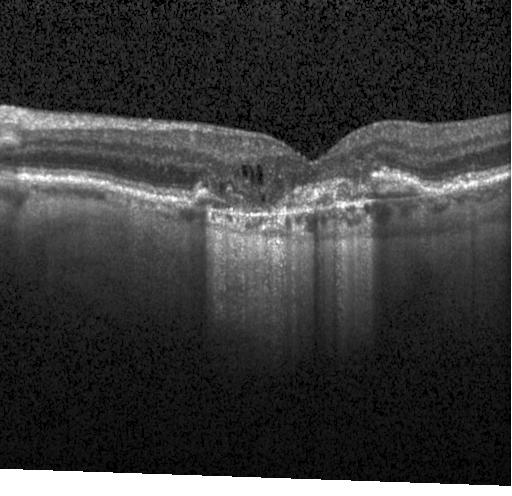
Horizontal scan through the fovea · optical coherence tomography B-scan. Impression: a choroidal neovascular membrane.